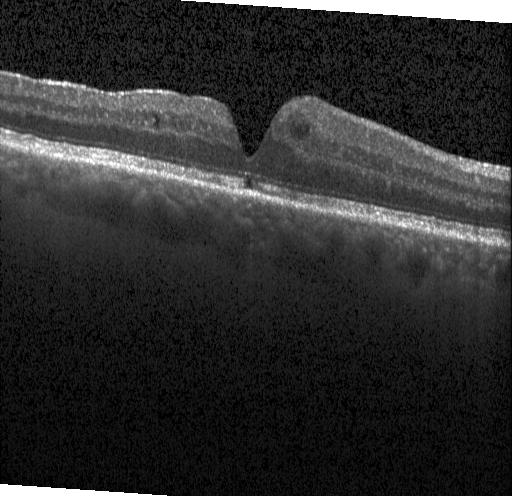
Retinal OCT B-scan. Finding: diabetic macular edema (DME).